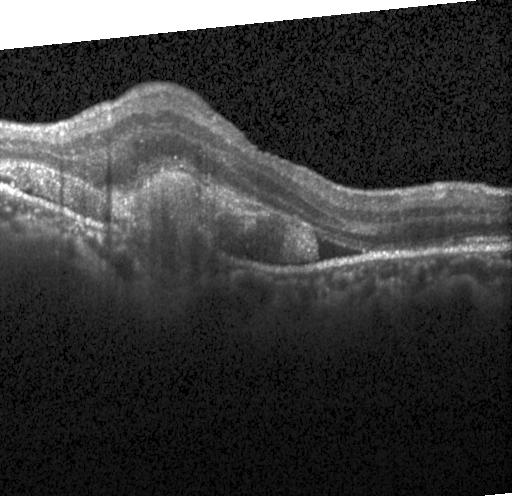
OCT finding: choroidal neovascularization.